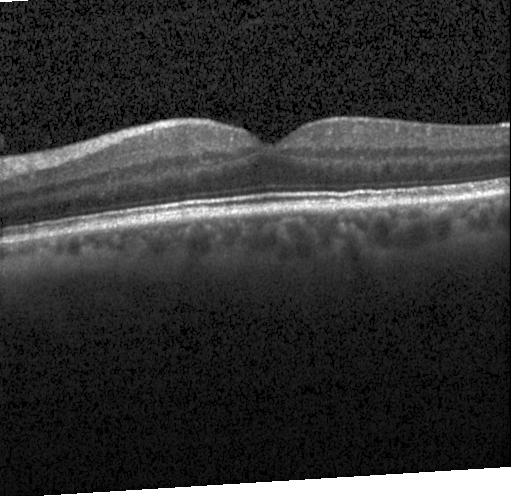 Optical coherence tomography B-scan — No evidence of CNV, DME, or drusen.